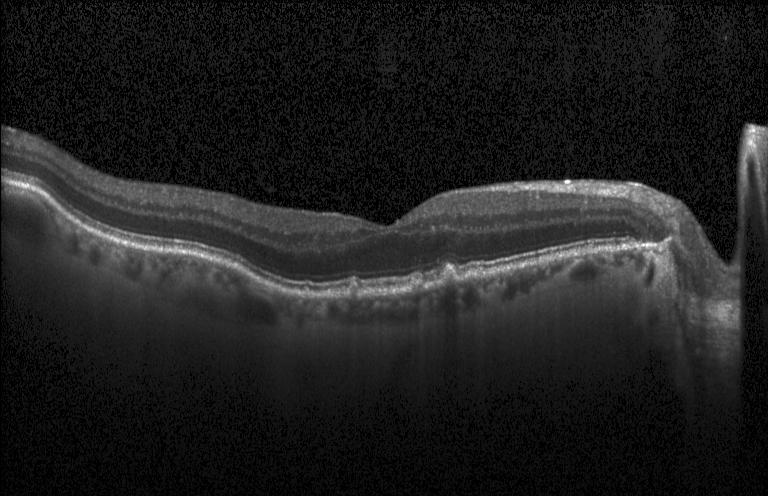 Retinal OCT cross-section · macular scan.
Dx: sub-RPE drusenoid deposits.